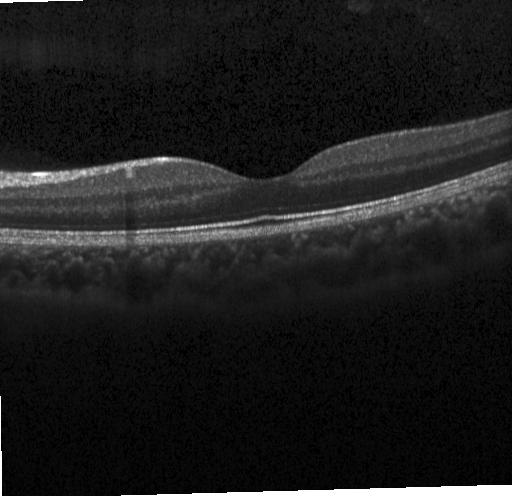

Spectral-domain optical coherence tomography. Retinal OCT cross-section. Heidelberg Spectralis OCT system — Diagnosis: no evidence of CNV, DME, or drusen.